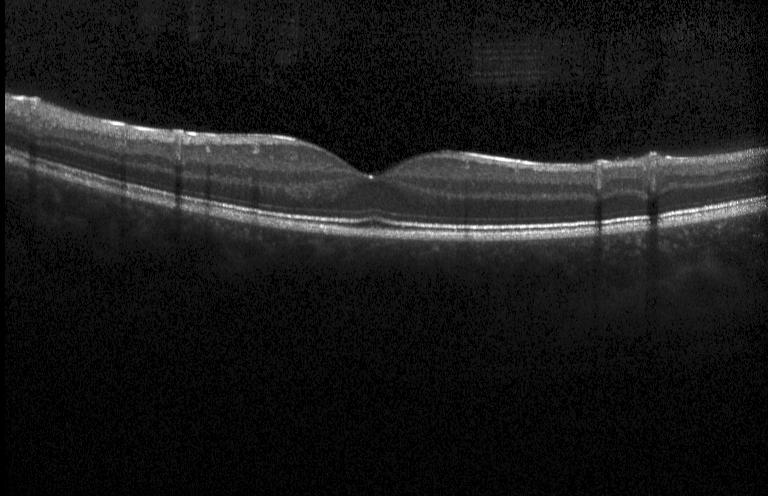 Spectral-domain optical coherence tomography, retinal OCT B-scan, macular scan, Heidelberg Spectralis
Impression: no choroidal neovascularization, diabetic macular edema, or drusen.